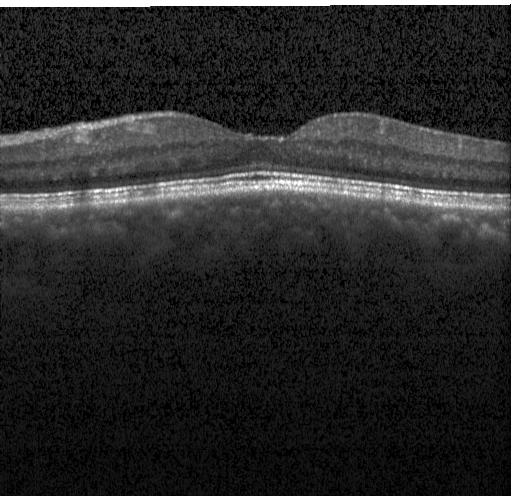 Optical coherence tomography B-scan; centered on the fovea — OCT finding: no choroidal neovascularization, diabetic macular edema, or drusen.